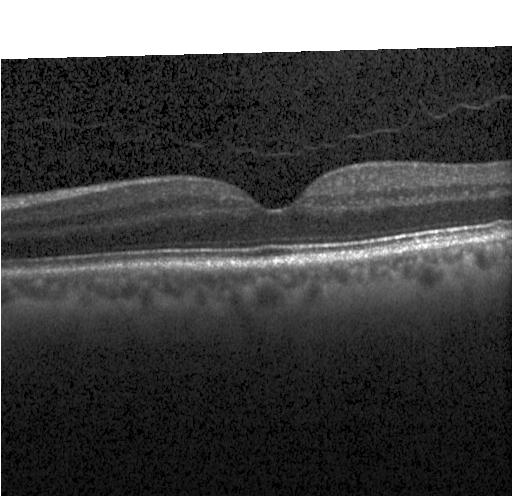

Finding: no choroidal neovascularization, no diabetic macular edema, and no drusen.